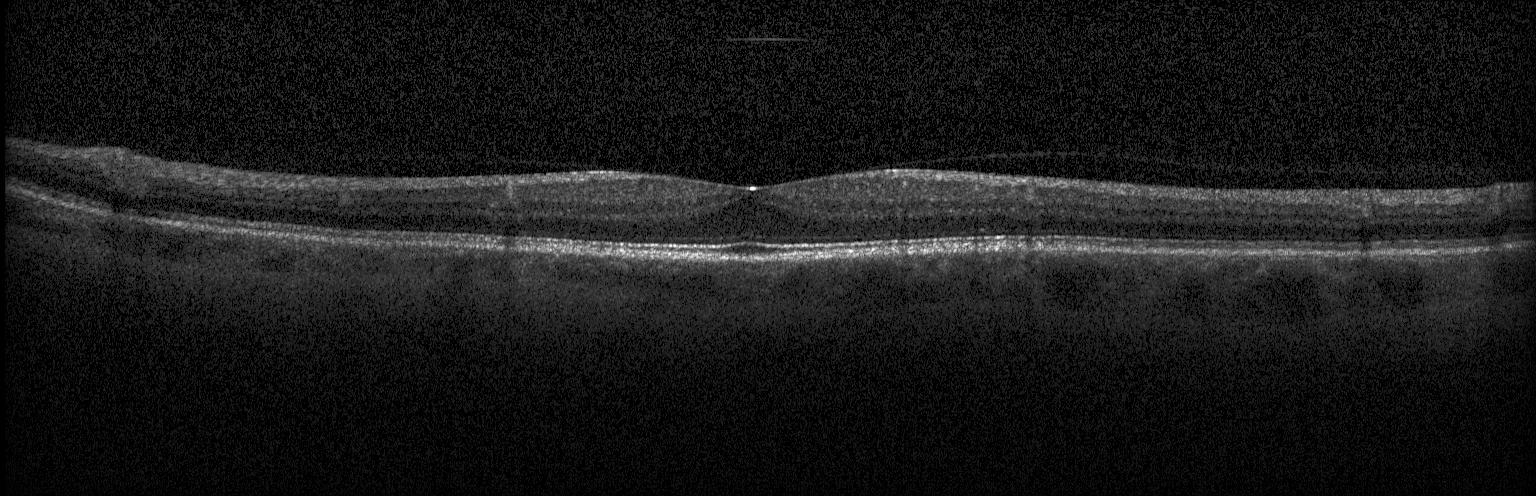

SD-OCT. Centered on the fovea. Optical coherence tomography B-scan.
Finding: no choroidal neovascularization, diabetic macular edema, or drusen.